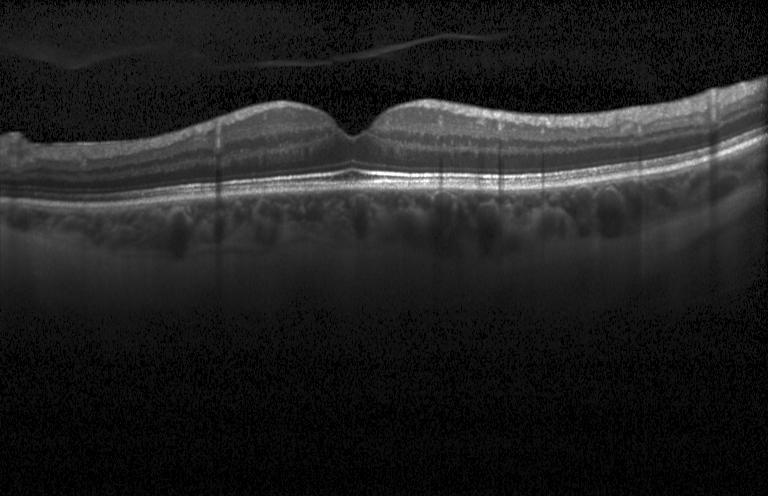

Instrument: Heidelberg Spectralis · optical coherence tomography scan · through the macula. Assessment: no choroidal neovascularization, diabetic macular edema, or drusen.